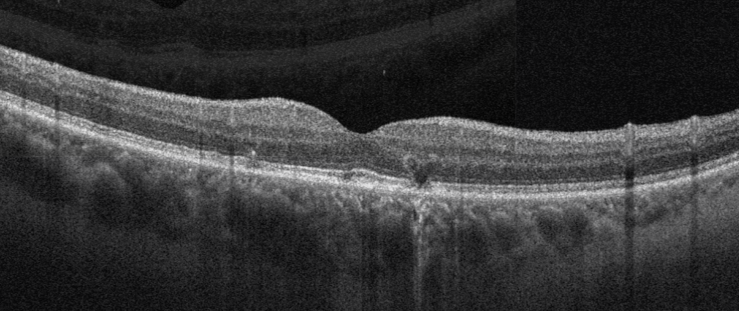 Retinal OCT B-scan. Fovea-centered. Acquired on an Optovue Avanti RTVue XR. Impression: age-related macular degeneration.